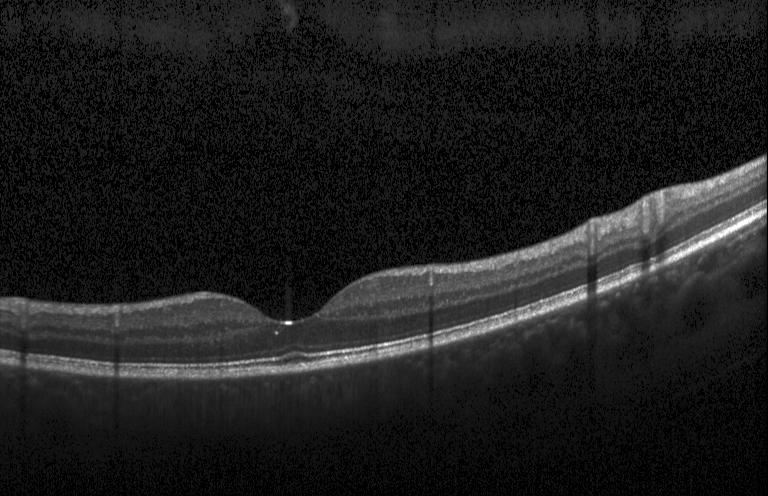
Optical coherence tomography B-scan.
Impression: no evidence of choroidal neovascularization, diabetic macular edema, or drusen.